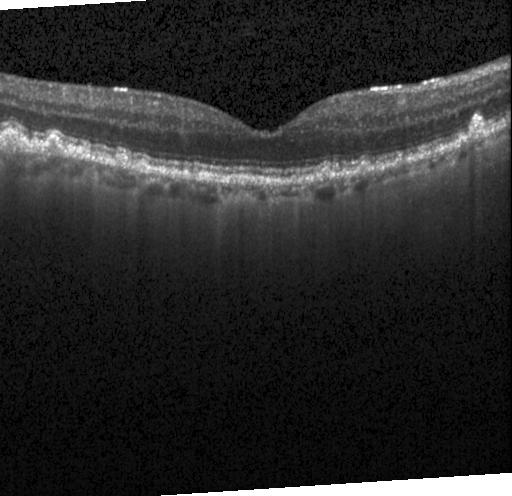 OCT line scan.
OCT finding: drusen.